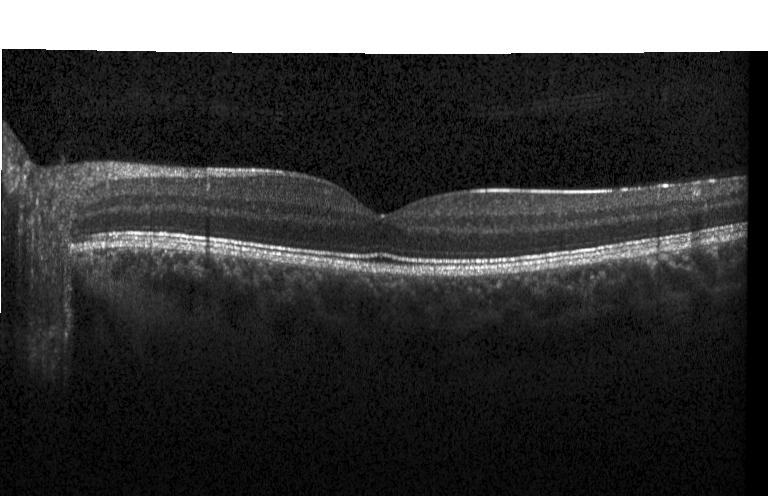 Fovea-centered; Heidelberg Spectralis OCT system; optical coherence tomography B-scan. No evidence of choroidal neovascularization, diabetic macular edema, or drusen.